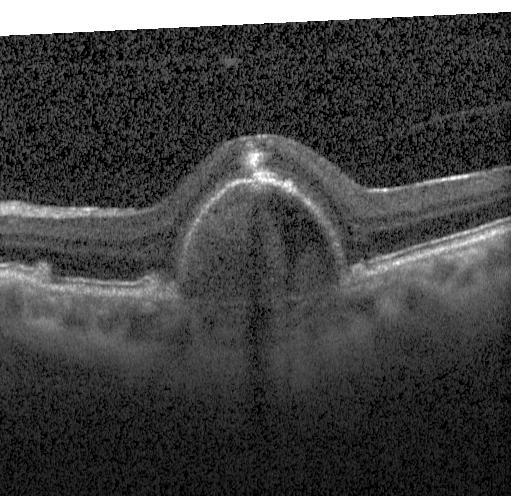 Diagnosis: a choroidal neovascular membrane.